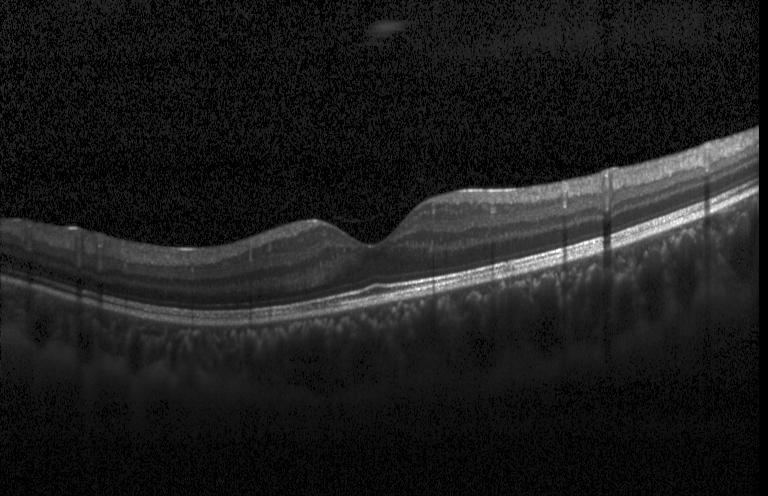

Impression: no choroidal neovascularization, no diabetic macular edema, and no drusen.